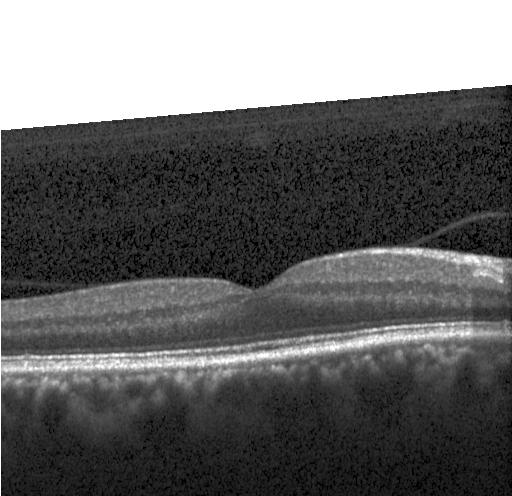
The scan shows neither choroidal neovascularization, diabetic macular edema, nor drusen.